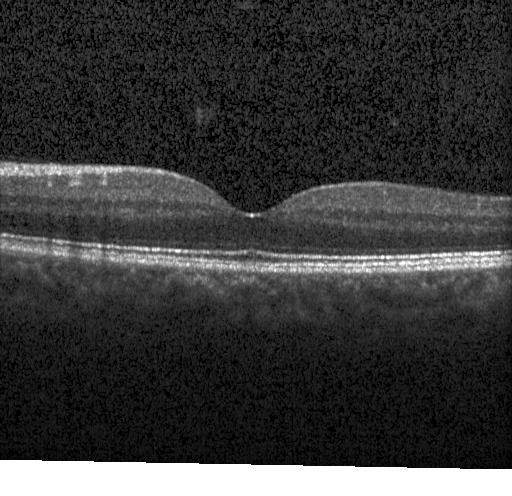 Diagnosis: no choroidal neovascularization, diabetic macular edema, or drusen.